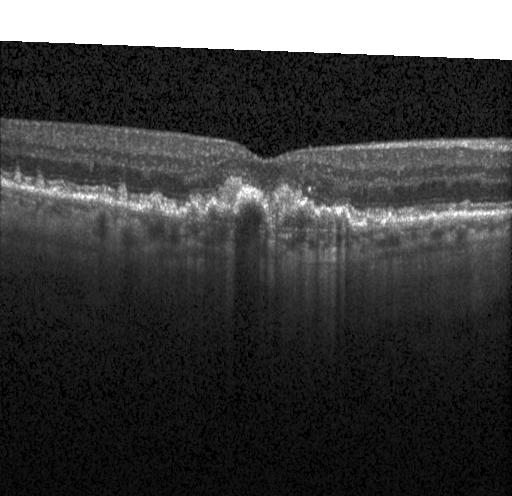 Optical coherence tomography scan — Diagnosis: a choroidal neovascular membrane.